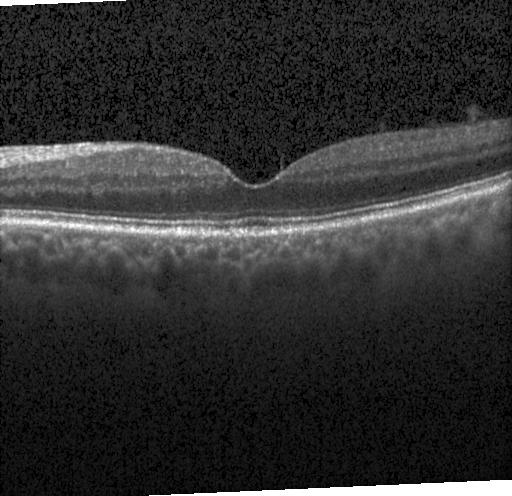 Retinal OCT cross-section
Impression: neither choroidal neovascularization, diabetic macular edema, nor drusen.